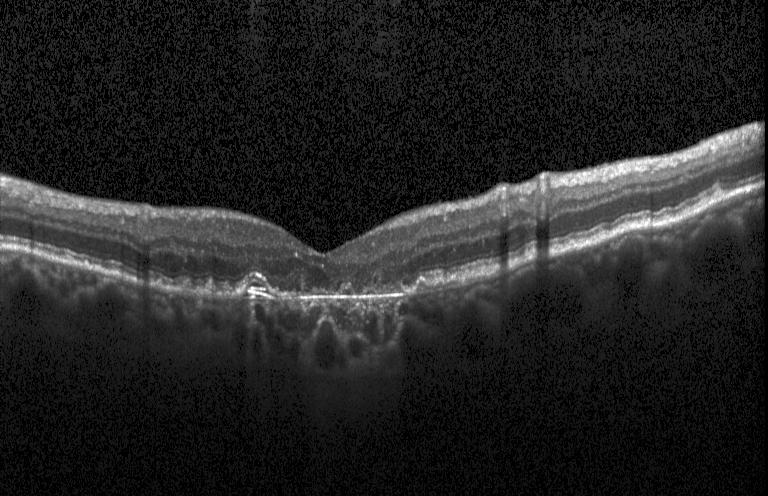
Diagnosis: choroidal neovascularization.